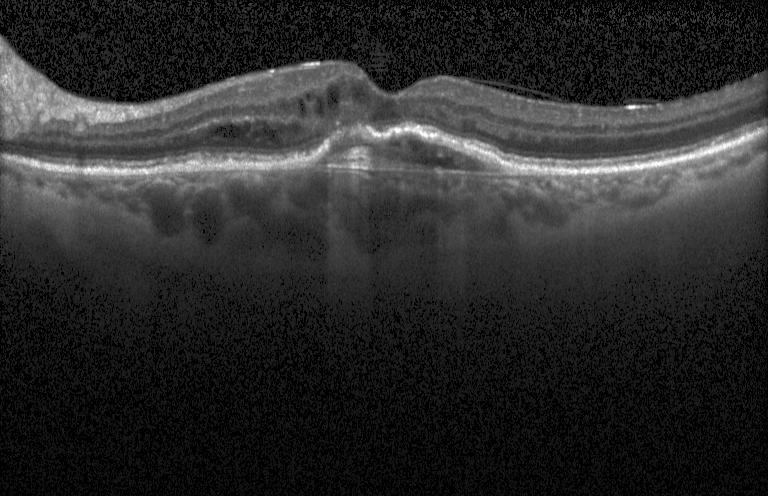 Retinal OCT cross-section, centered on the fovea, instrument: Heidelberg Spectralis, spectral-domain OCT
This B-scan demonstrates CNV.